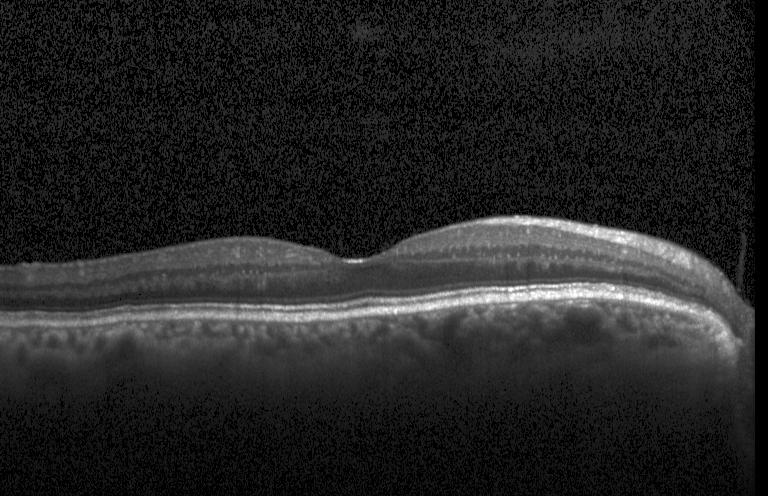
Macular scan; optical coherence tomography B-scan; acquired on a Heidelberg Spectralis; spectral-domain OCT — Assessment: no evidence of choroidal neovascularization, diabetic macular edema, or drusen.